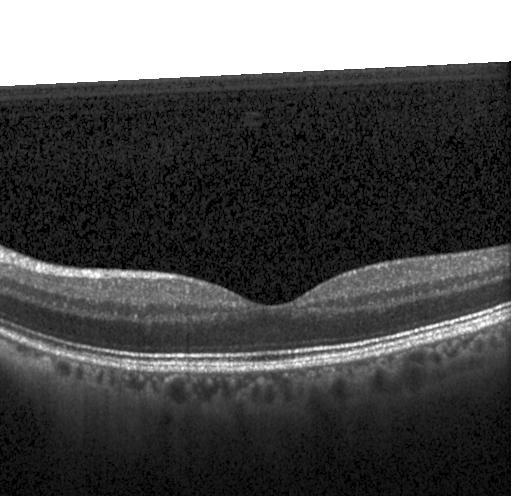 Diagnosis: no CNV, no DME, and no drusen.